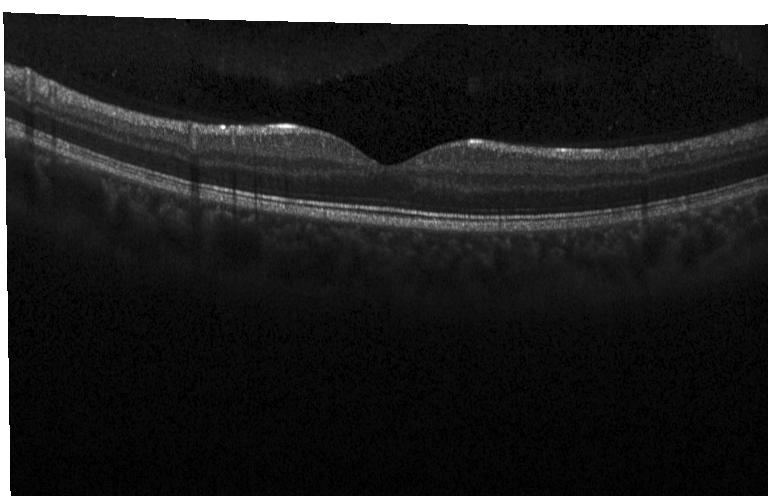

Retinal OCT B-scan — Finding: no evidence of choroidal neovascularization, diabetic macular edema, or drusen.